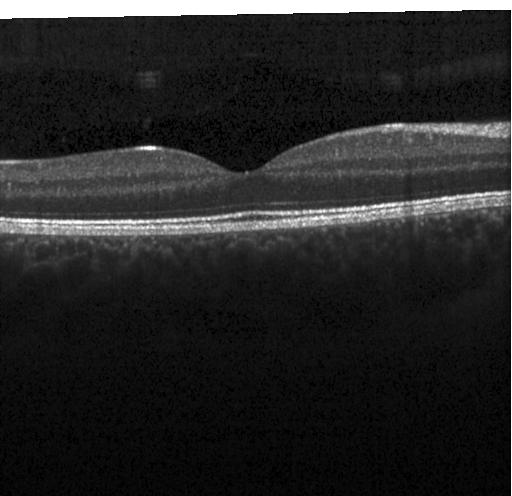
Retinal OCT cross-section · macular scan · Heidelberg Spectralis OCT system · spectral-domain OCT. Macular OCT: no choroidal neovascularization, no diabetic macular edema, and no drusen.